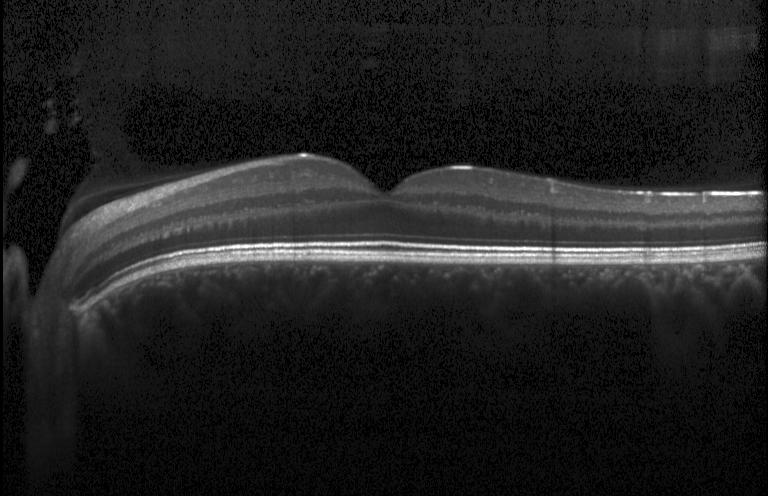 Through the macula, spectral-domain OCT, OCT B-scan, Heidelberg Spectralis
Dx: no evidence of choroidal neovascularization, diabetic macular edema, or drusen.